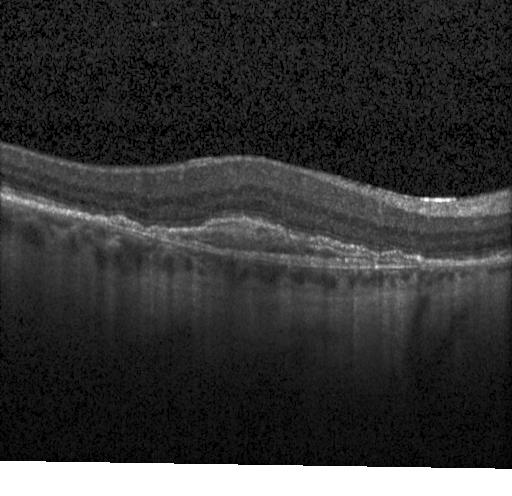 Retinal OCT cross-section showing a choroidal neovascular membrane.